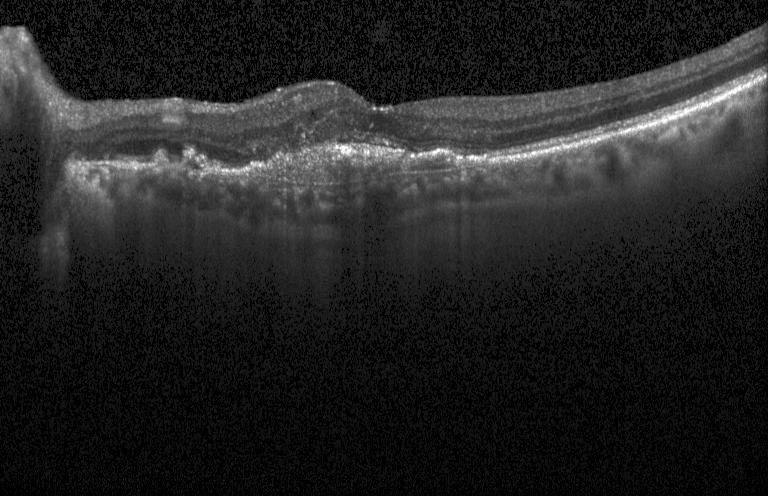
Centered on the fovea. Optical coherence tomography scan. Spectral-domain OCT — OCT finding: a choroidal neovascular membrane.